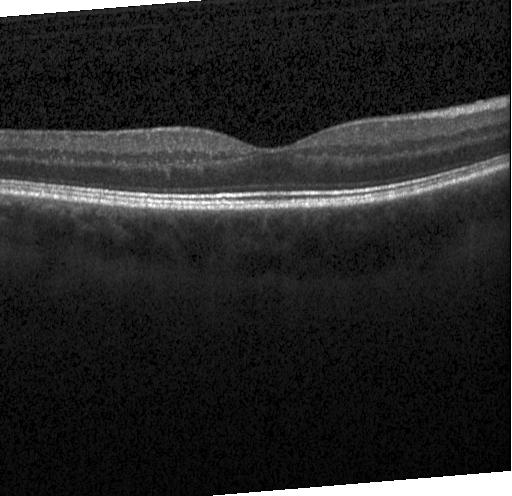
Spectral-domain OCT. Fovea-centered. Optical coherence tomography B-scan.
The scan shows neither choroidal neovascularization, diabetic macular edema, nor drusen.